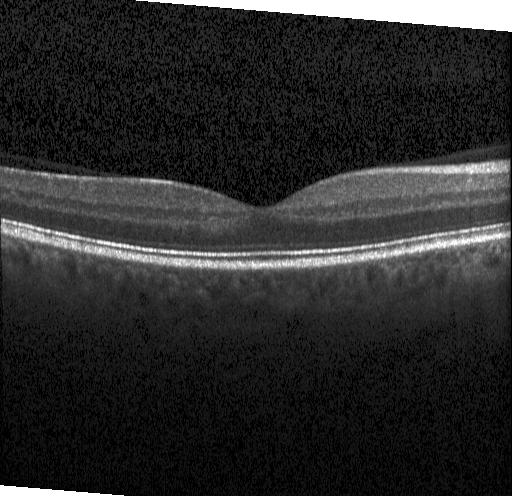 Impression: no choroidal neovascularization, no diabetic macular edema, and no drusen.